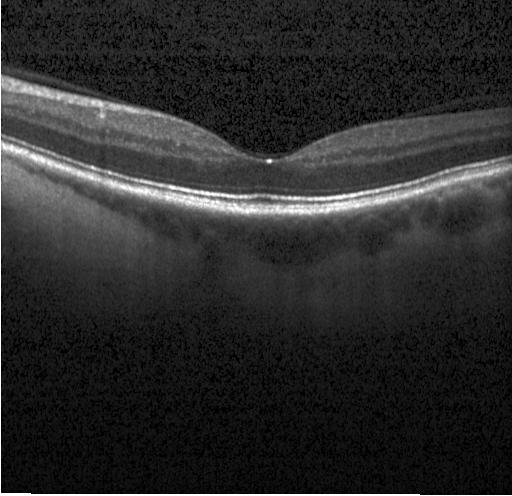
Optical coherence tomography B-scan.
Finding: no evidence of choroidal neovascularization, diabetic macular edema, or drusen.